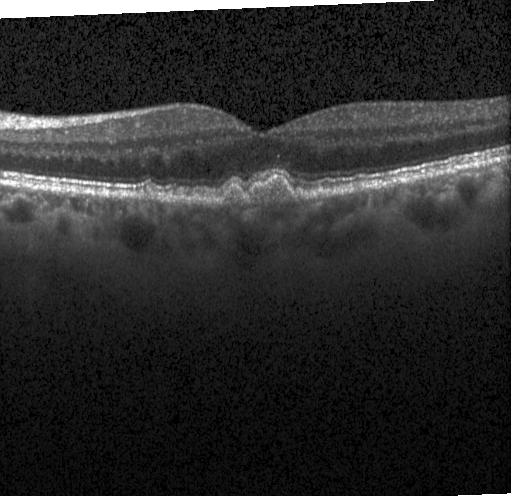

Acquired on a Heidelberg Spectralis. Spectral-domain optical coherence tomography. Retinal OCT B-scan — Drusen.